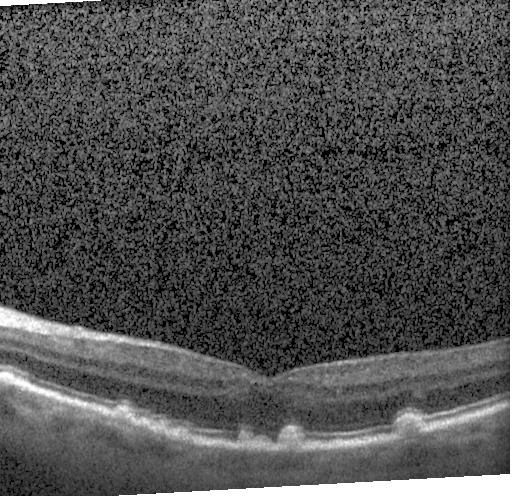

Macular OCT demonstrating drusen.